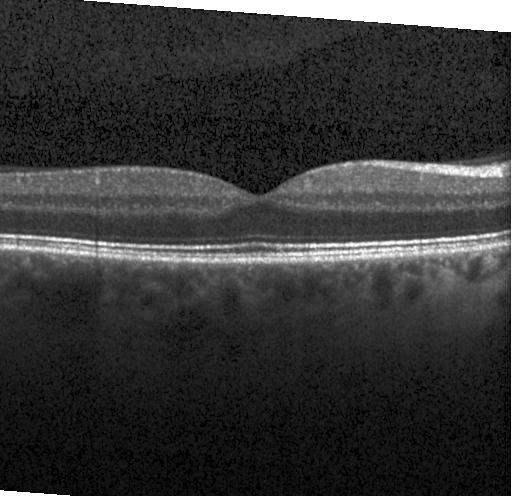 Retinal OCT cross-section; acquired on a Heidelberg Spectralis. Impression: no choroidal neovascularization, no diabetic macular edema, and no drusen.